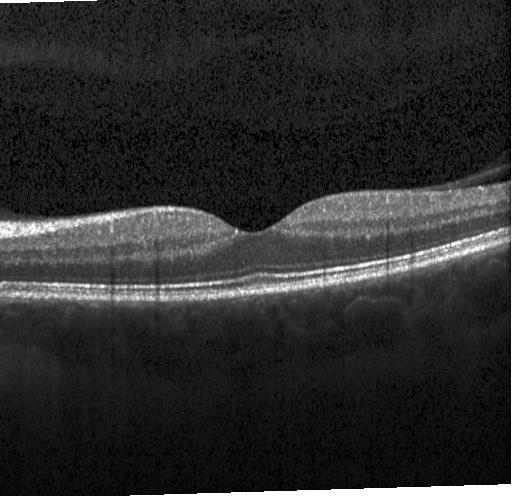

Spectral-domain optical coherence tomography, macular scan, acquired on a Heidelberg Spectralis, OCT B-scan — No choroidal neovascularization, diabetic macular edema, or drusen.